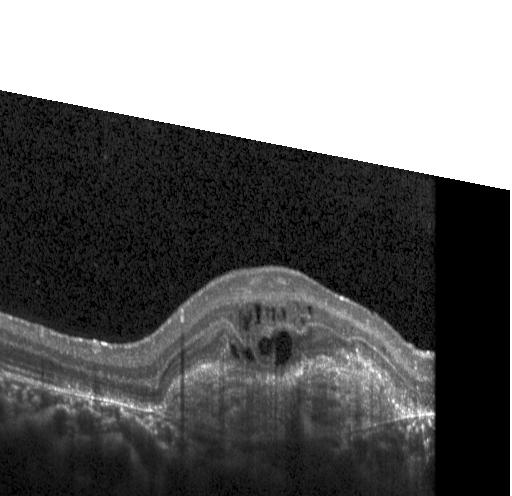
Macular OCT demonstrating a choroidal neovascular membrane.